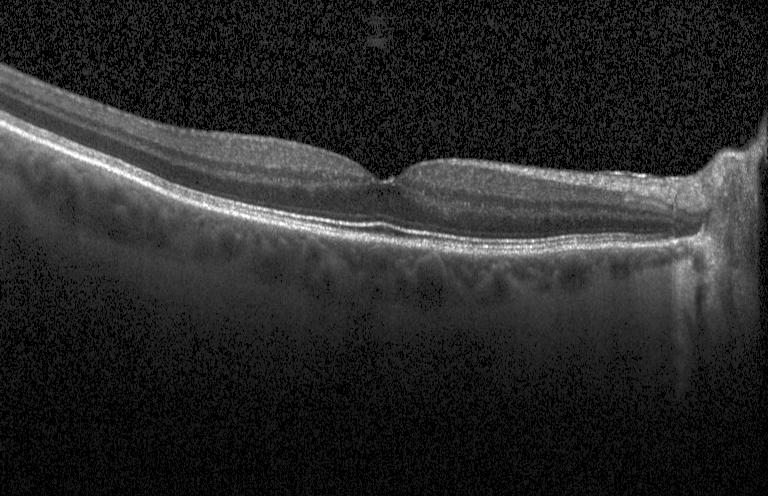 OCT line scan · fovea-centered · SD-OCT. Impression: no evidence of CNV, DME, or drusen.